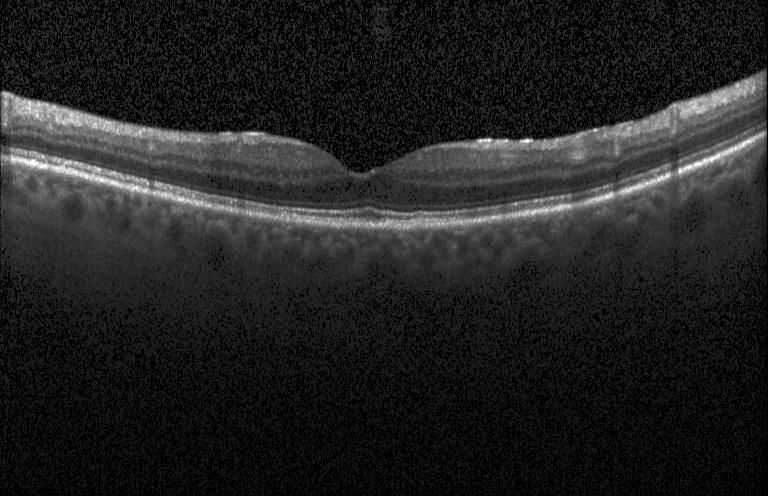

SD-OCT. OCT B-scan.
No choroidal neovascularization, diabetic macular edema, or drusen.